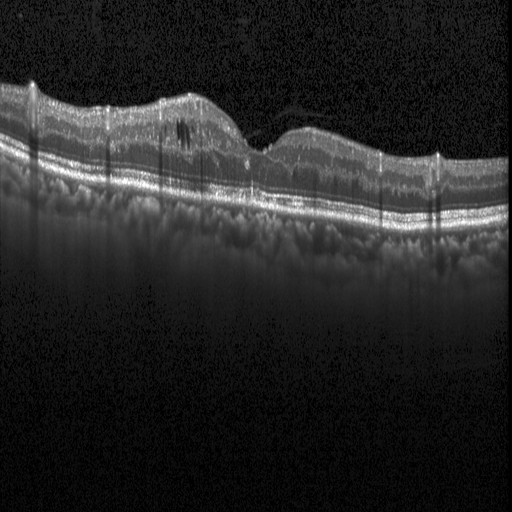 Acquired on a Heidelberg Spectralis · OCT line scan · macular scan · spectral-domain OCT — OCT finding: diabetic macular edema.